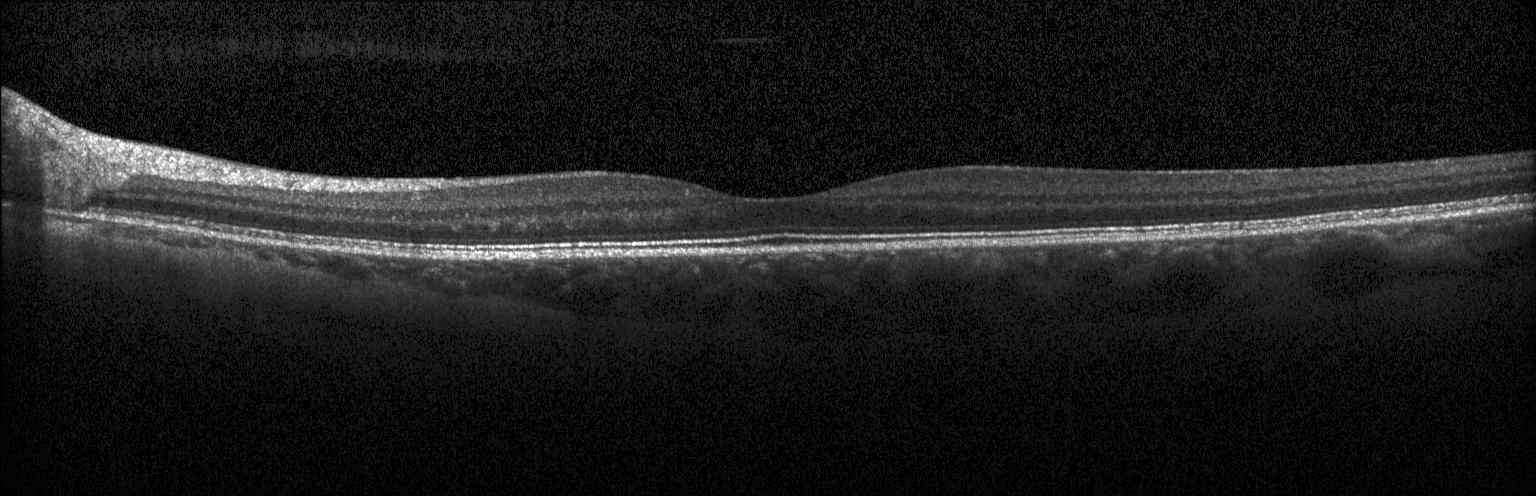 Spectral-domain OCT. Heidelberg Spectralis. OCT line scan. Centered on the fovea — Neither CNV, DME, nor drusen.